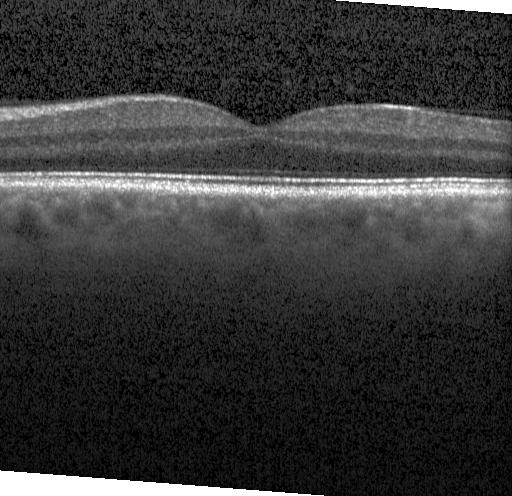 Instrument: Heidelberg Spectralis. Spectral-domain optical coherence tomography. Retinal OCT B-scan. Macular scan. Finding: neither choroidal neovascularization, diabetic macular edema, nor drusen.